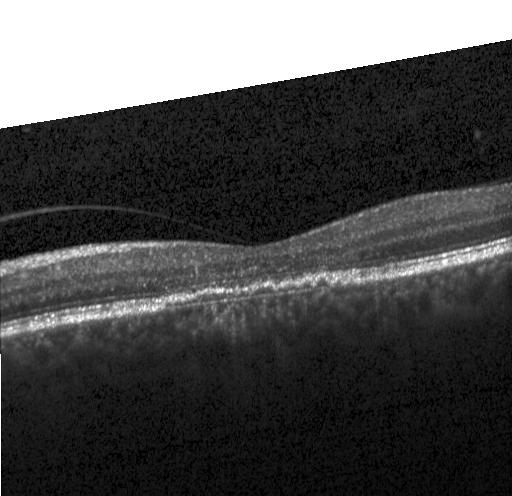

Spectral-domain optical coherence tomography · through the macula · retinal OCT cross-section · acquired on a Heidelberg Spectralis
Macular OCT: choroidal neovascularization (CNV).